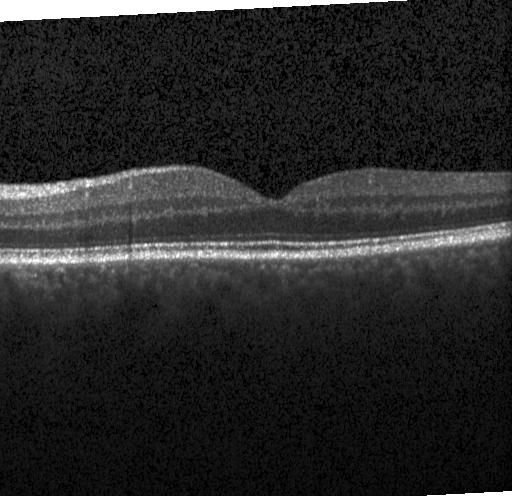

Optical coherence tomography scan — Macular OCT: no evidence of choroidal neovascularization, diabetic macular edema, or drusen.